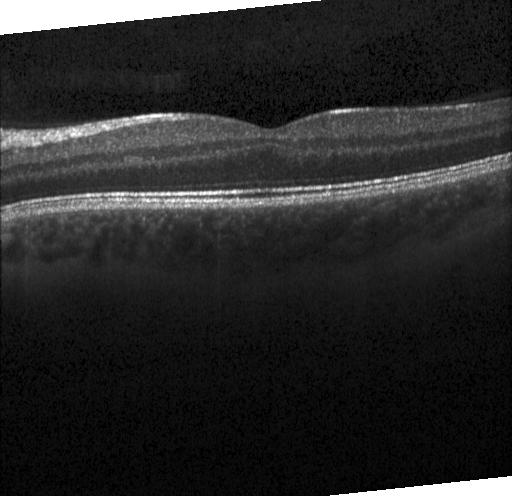

Retinal OCT cross-section. Impression: no evidence of choroidal neovascularization, diabetic macular edema, or drusen.